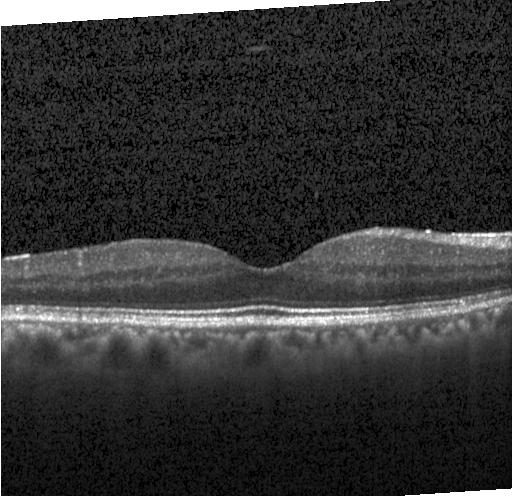

Optical coherence tomography scan; Heidelberg Spectralis.
Assessment: no choroidal neovascularization, no diabetic macular edema, and no drusen.